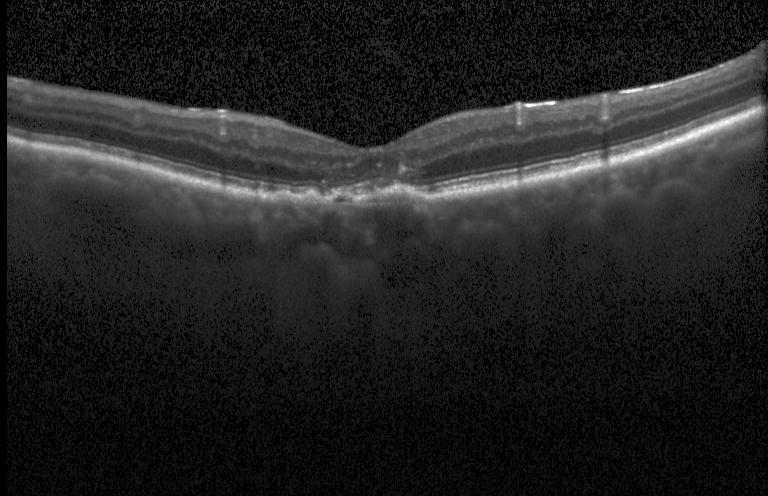
Retinal OCT B-scan. This B-scan demonstrates a choroidal neovascular membrane.